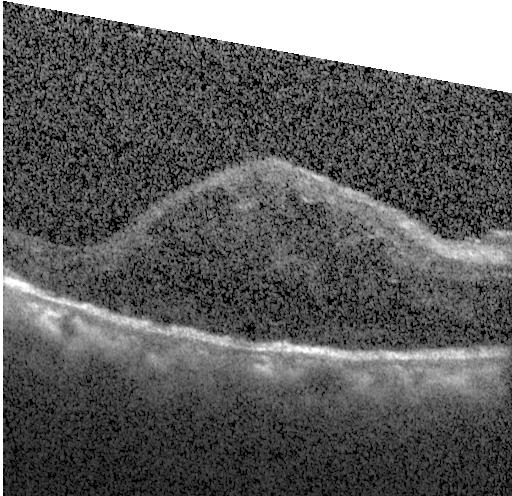
Optical coherence tomography scan; spectral-domain optical coherence tomography.
The scan shows diabetic macular edema.